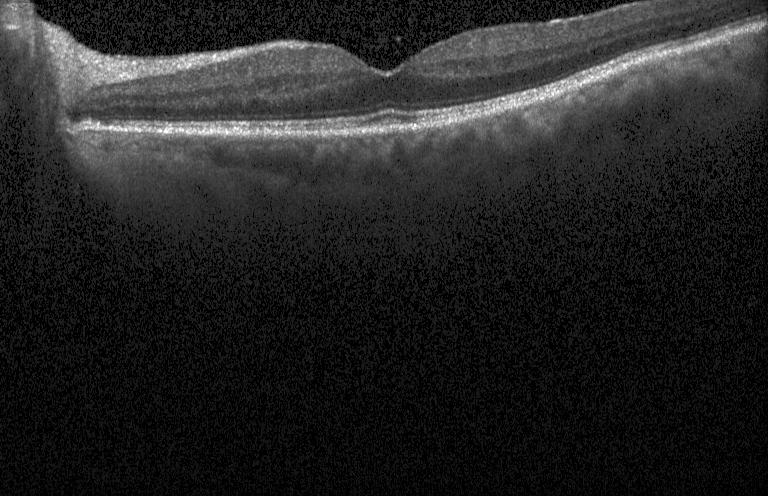 This B-scan demonstrates no choroidal neovascularization, diabetic macular edema, or drusen.